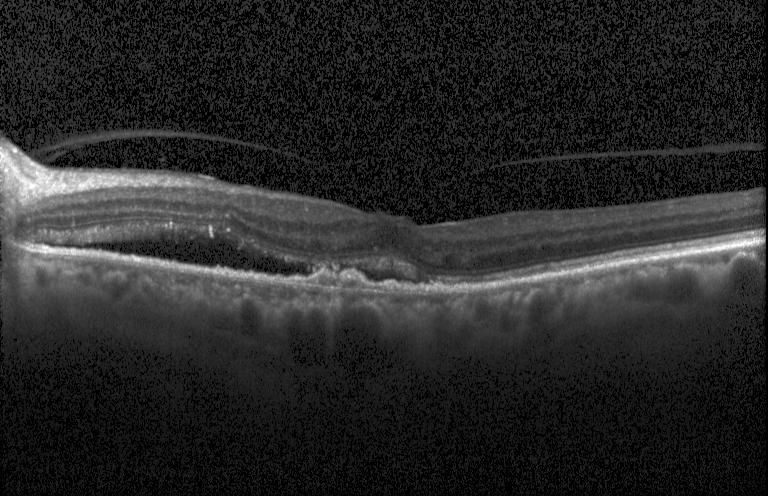
Macular scan · spectral-domain optical coherence tomography · retinal OCT B-scan
OCT finding: a choroidal neovascular membrane.